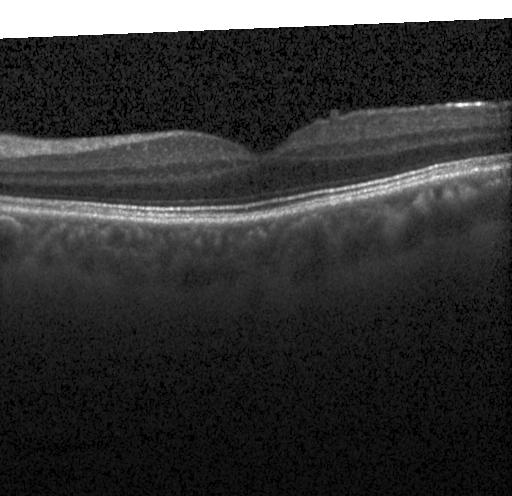
OCT B-scan — Impression: no choroidal neovascularization, no diabetic macular edema, and no drusen.